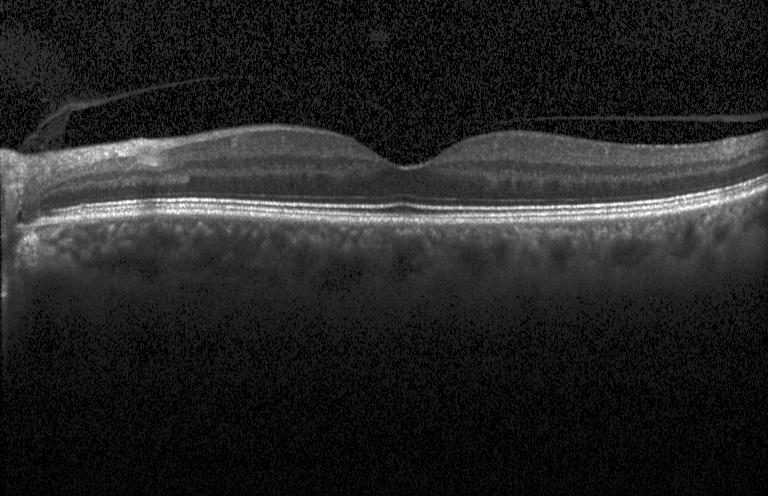

Spectral-domain optical coherence tomography, optical coherence tomography B-scan.
OCT finding: no CNV, no DME, and no drusen.